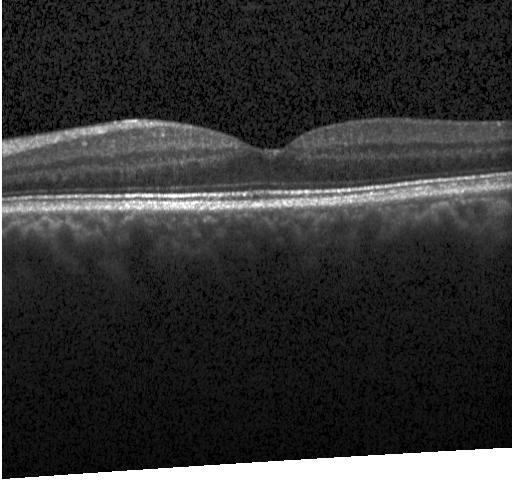
Impression: no choroidal neovascularization, diabetic macular edema, or drusen.